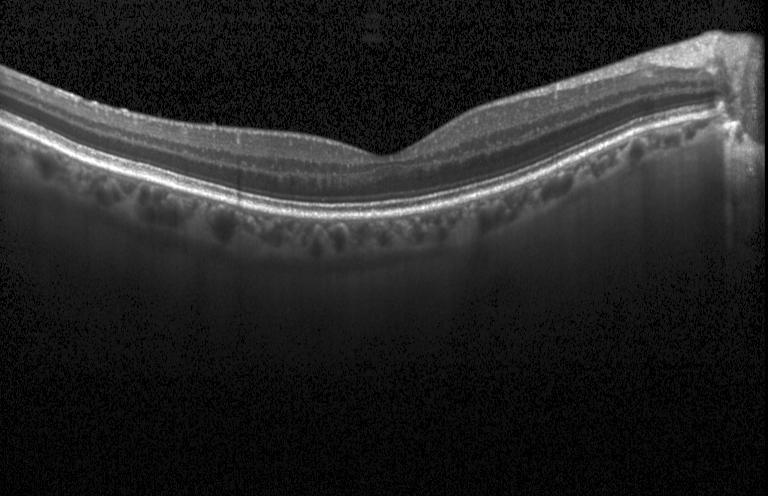
Heidelberg Spectralis · spectral-domain OCT · optical coherence tomography scan · macular scan — Finding: neither choroidal neovascularization, diabetic macular edema, nor drusen.